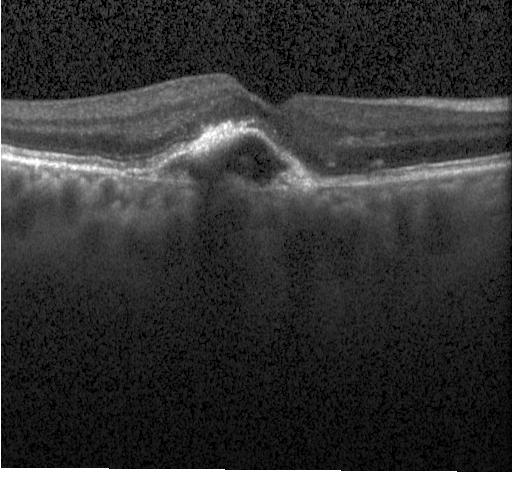

Optical coherence tomography B-scan, horizontal scan through the fovea — OCT finding: CNV.